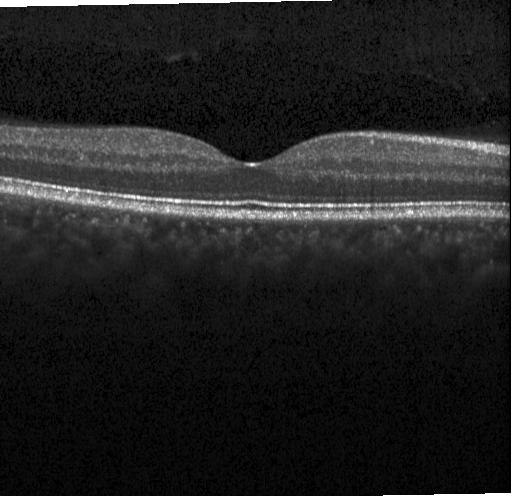

OCT B-scan. Macular scan.
No choroidal neovascularization, diabetic macular edema, or drusen.